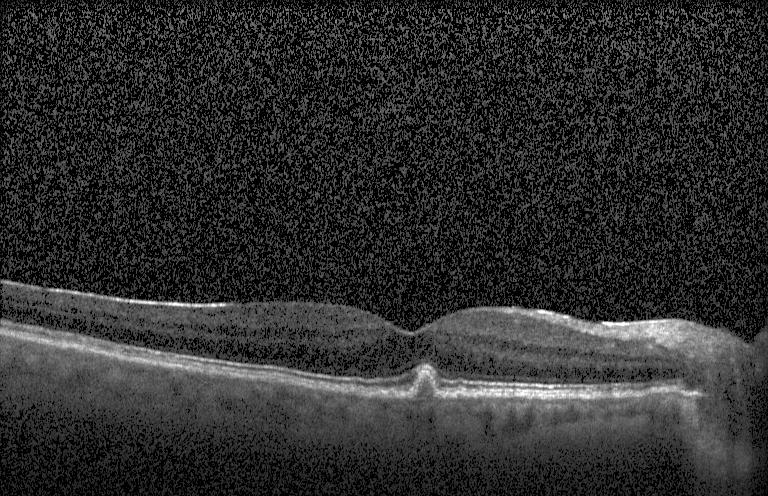
OCT B-scan · spectral-domain OCT — Finding: multiple drusen.